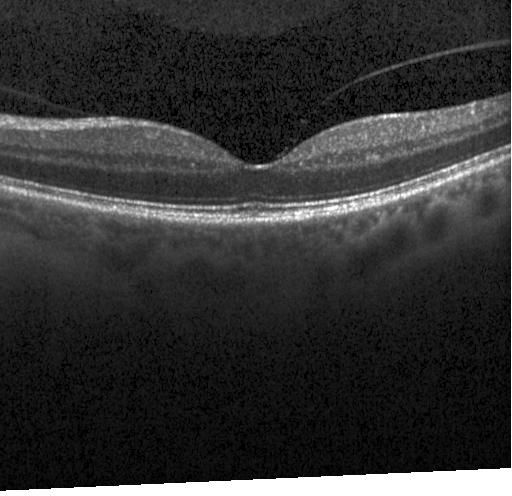

Impression: no choroidal neovascularization, no diabetic macular edema, and no drusen.